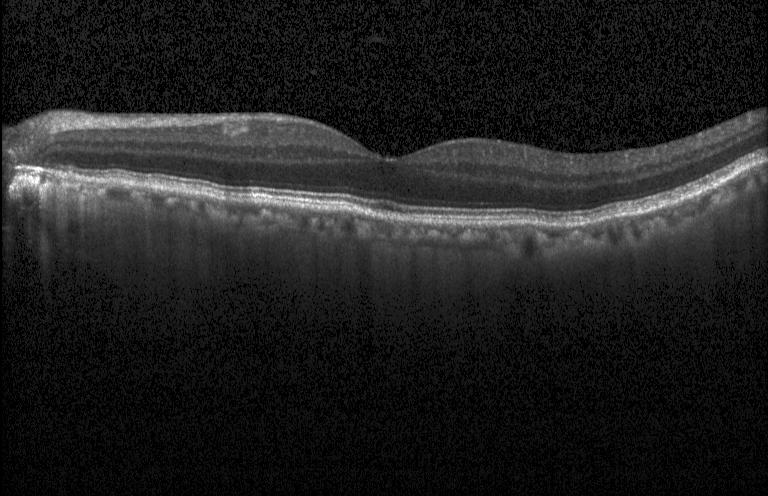
SD-OCT, acquired on a Heidelberg Spectralis, retinal OCT B-scan, macular scan — Finding: no CNV, DME, or drusen.